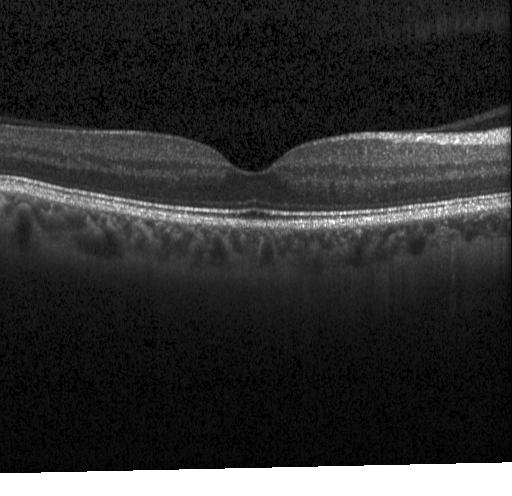 Finding: no CNV, DME, or drusen.